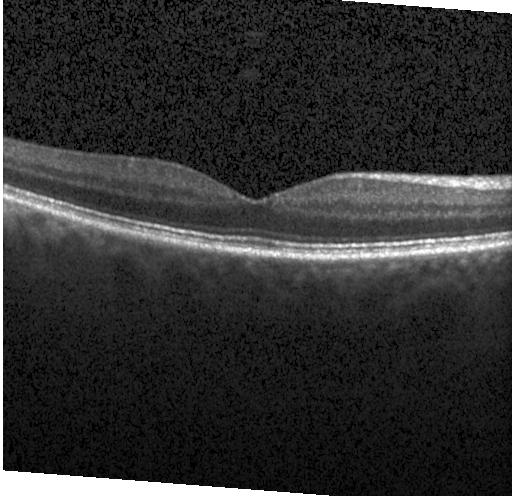

Optical coherence tomography B-scan — Finding: no CNV, no DME, and no drusen.